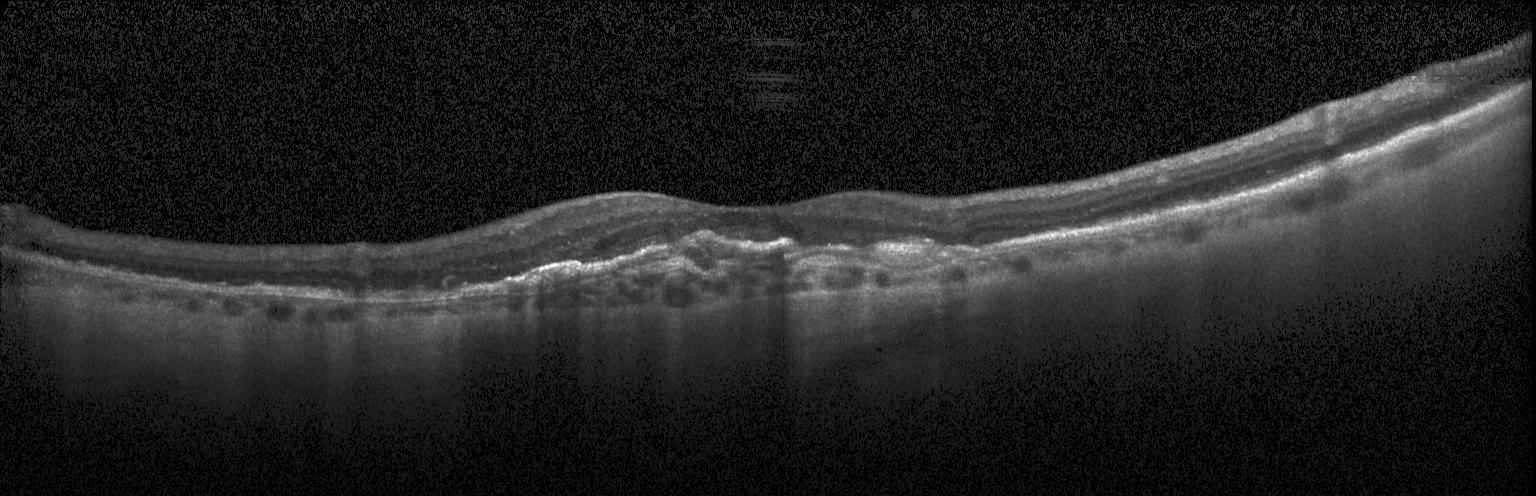
SD-OCT. Retinal OCT B-scan. The scan shows CNV.